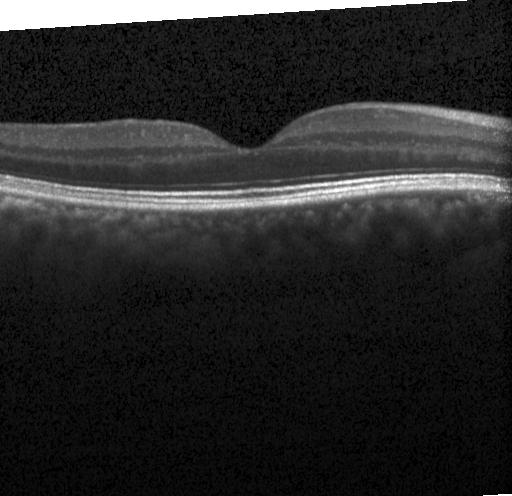
Retinal OCT B-scan.
The scan shows no evidence of choroidal neovascularization, diabetic macular edema, or drusen.